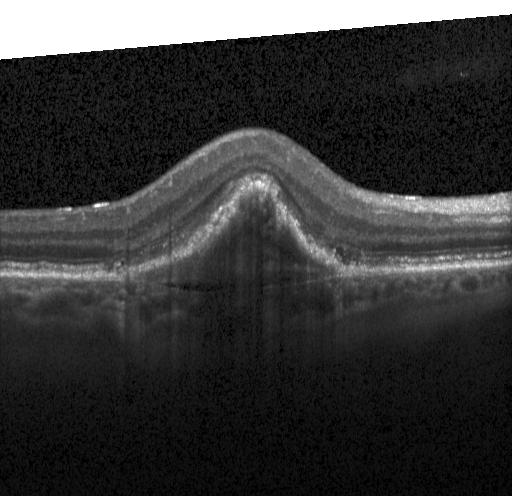

Spectral-domain OCT; horizontal scan through the fovea; retinal OCT cross-section.
Dx: CNV.